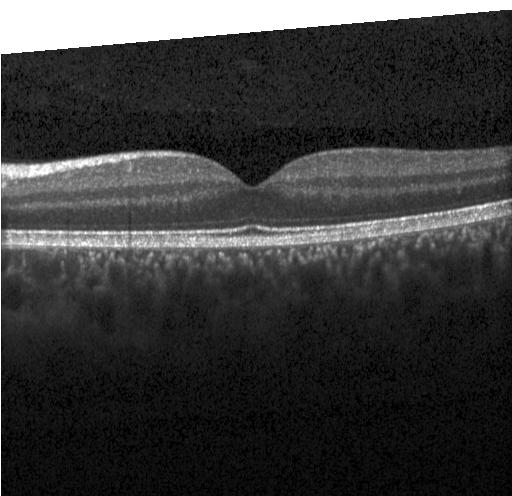

SD-OCT; retinal OCT cross-section. Impression: no evidence of choroidal neovascularization, diabetic macular edema, or drusen.